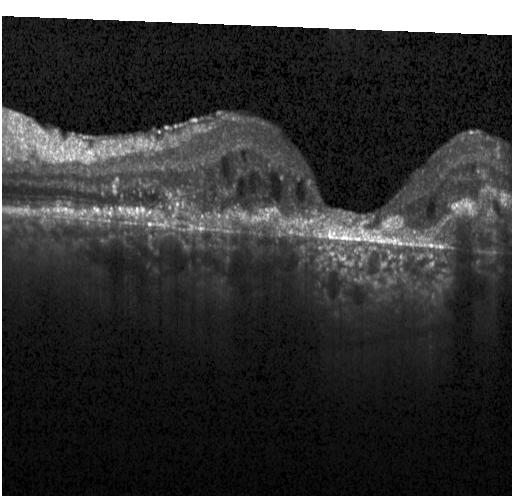 Dx: a choroidal neovascular membrane.